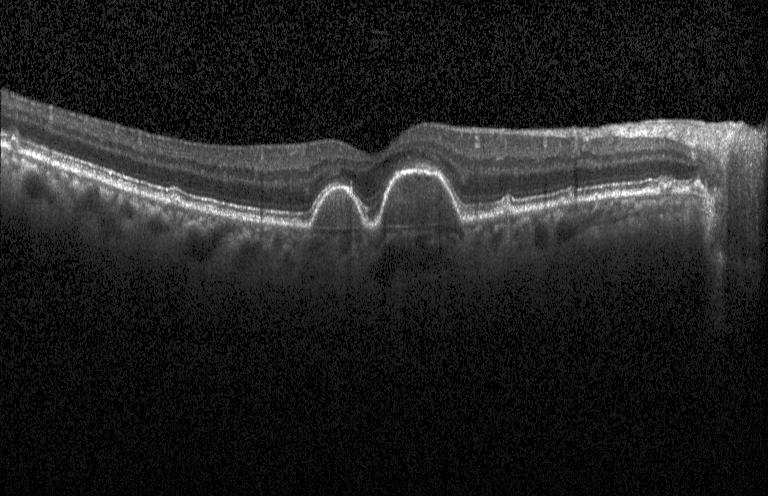

Heidelberg Spectralis OCT system; retinal OCT cross-section
Finding: multiple drusen.